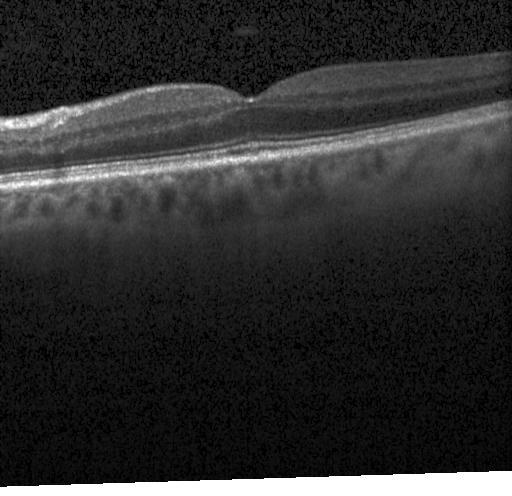
Spectral-domain OCT B-scan: no CNV, no DME, and no drusen.